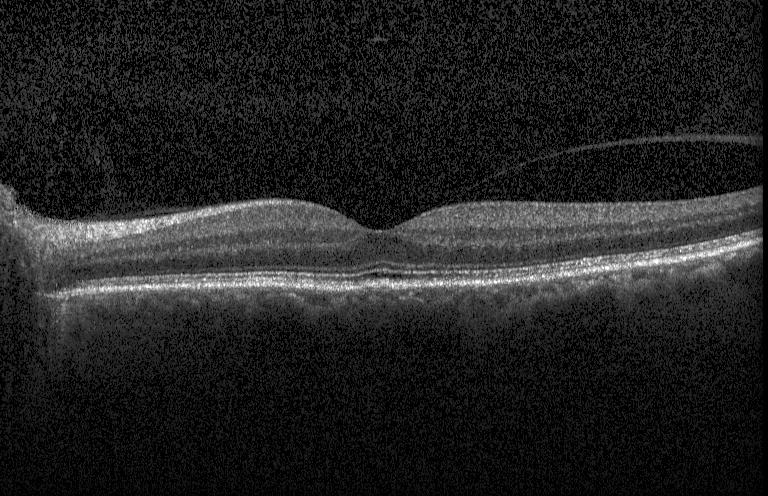 Retinal OCT B-scan · centered on the fovea · spectral-domain optical coherence tomography. Diagnosis: no choroidal neovascularization, diabetic macular edema, or drusen.